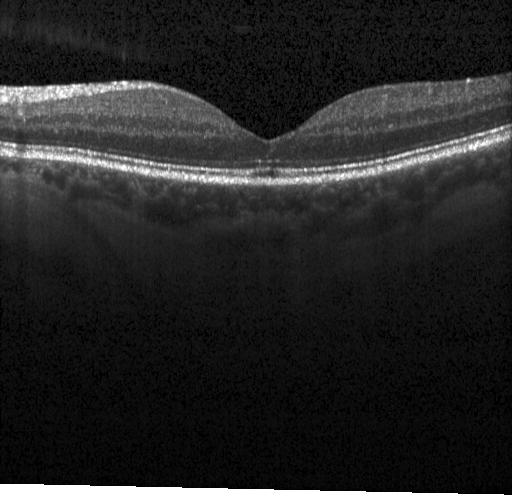
OCT B-scan. Diagnosis: no choroidal neovascularization, diabetic macular edema, or drusen.